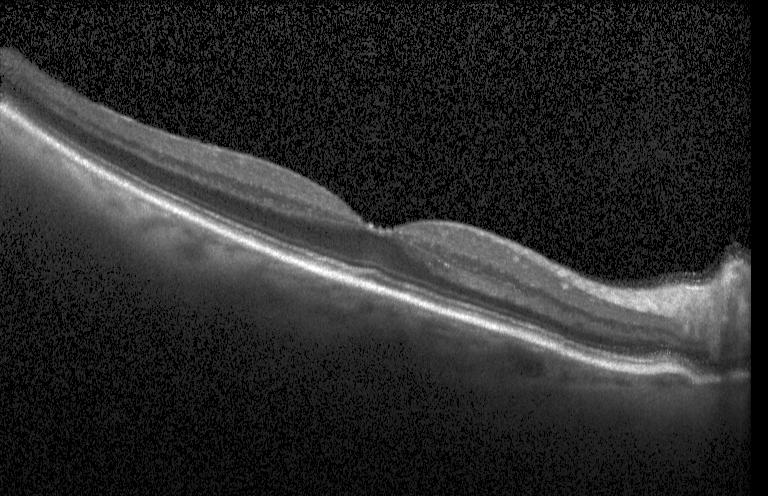
SD-OCT; retinal OCT cross-section; Heidelberg Spectralis
Macular OCT: no evidence of choroidal neovascularization, diabetic macular edema, or drusen.